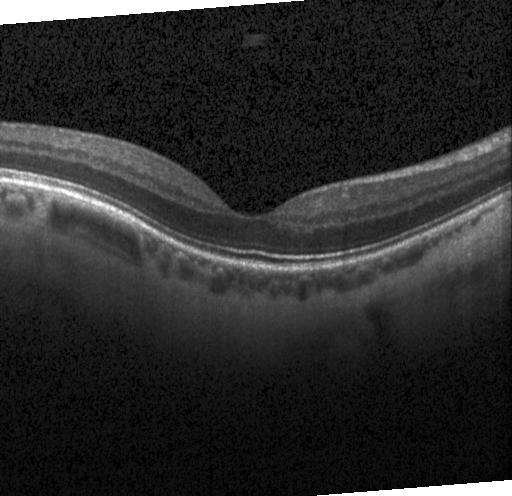

OCT line scan.
Diagnosis: no CNV, DME, or drusen.